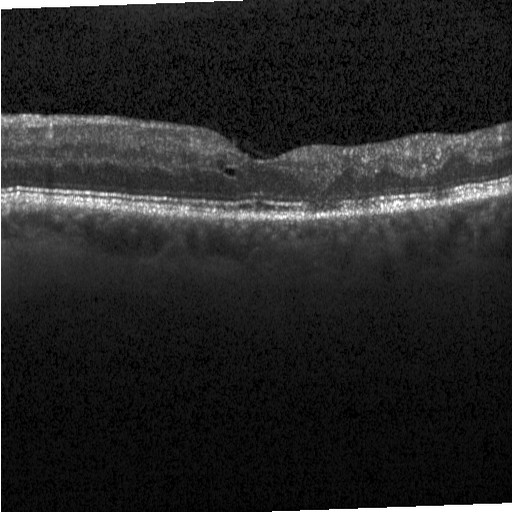 Optical coherence tomography B-scan, Heidelberg Spectralis, through the macula.
Diagnosis: diabetic macular edema (DME).